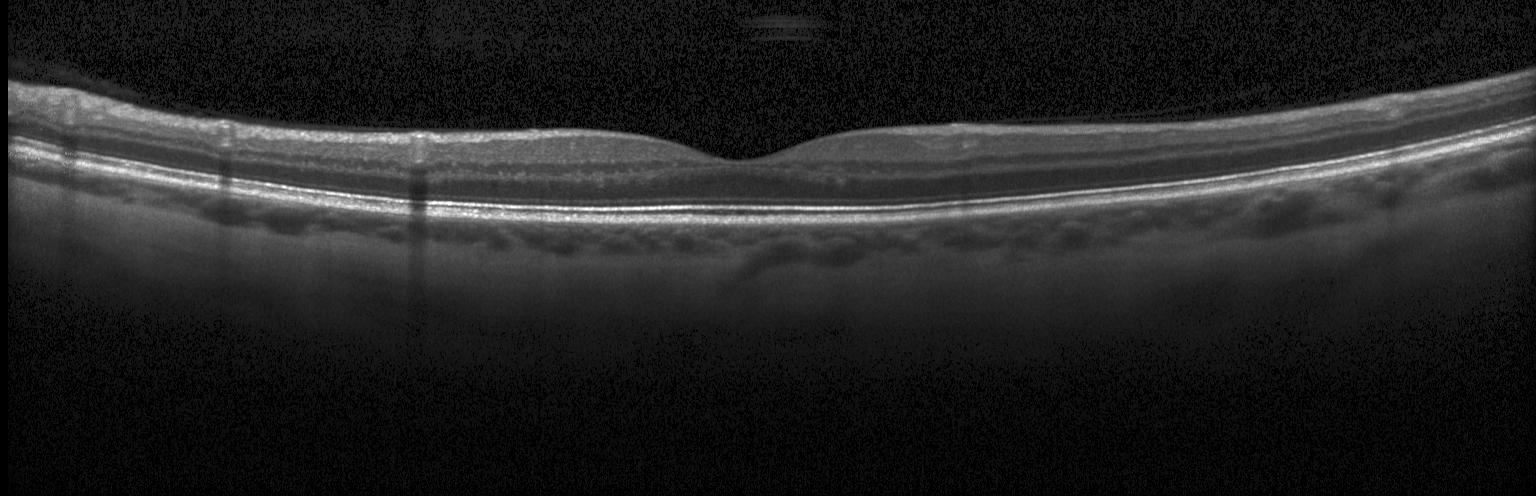 OCT B-scan.
This B-scan demonstrates no evidence of choroidal neovascularization, diabetic macular edema, or drusen.